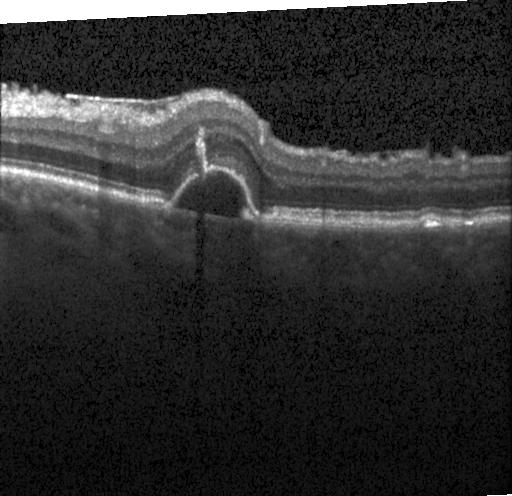

Retinal OCT B-scan, horizontal scan through the fovea — Impression: a choroidal neovascular membrane.